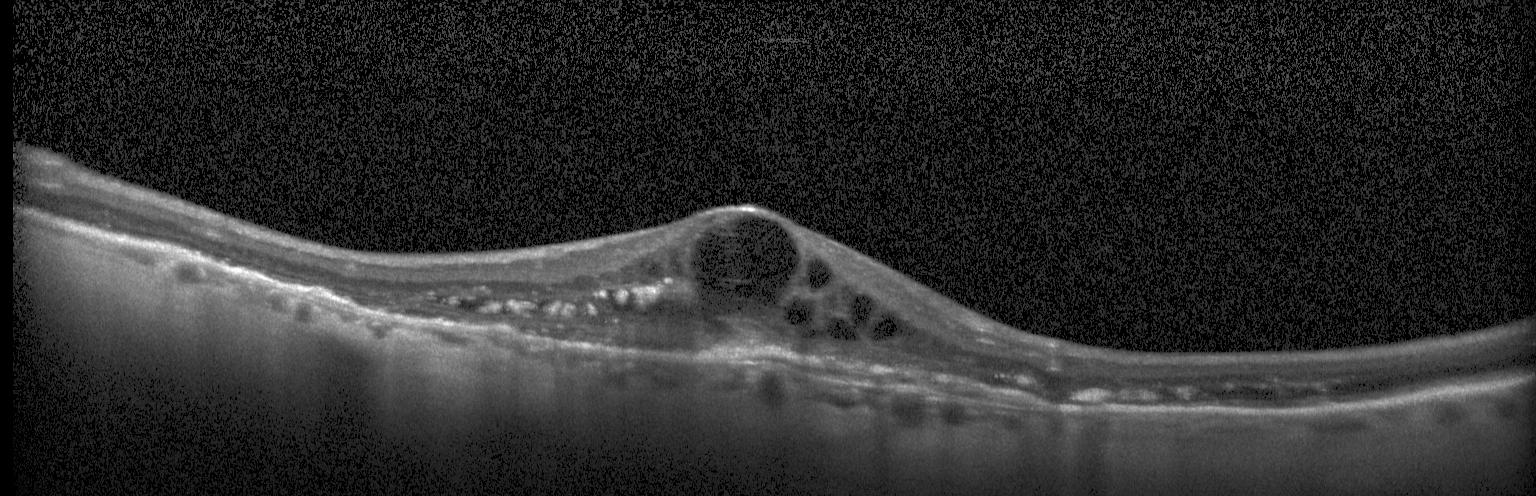 Impression: a choroidal neovascular membrane.